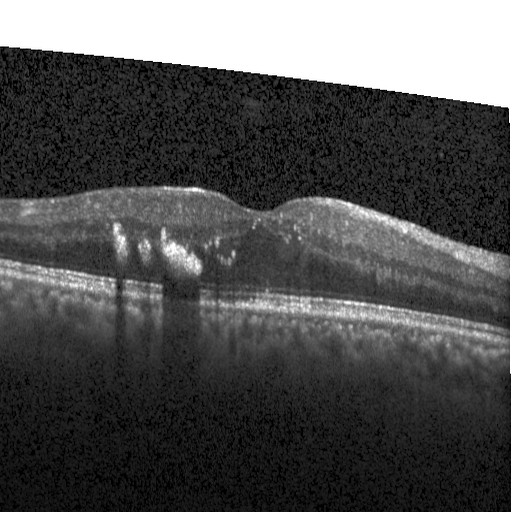

Spectral-domain optical coherence tomography · retinal OCT B-scan.
Finding: diabetic macular edema.